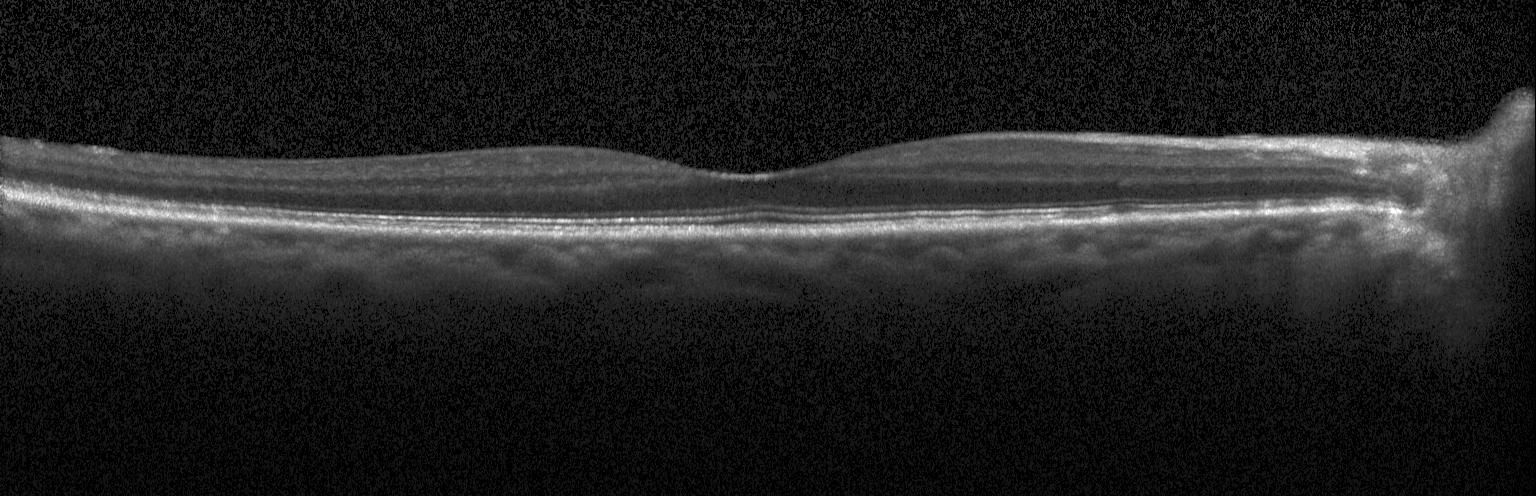 OCT line scan; acquired on a Heidelberg Spectralis — Diagnosis: no evidence of CNV, DME, or drusen.